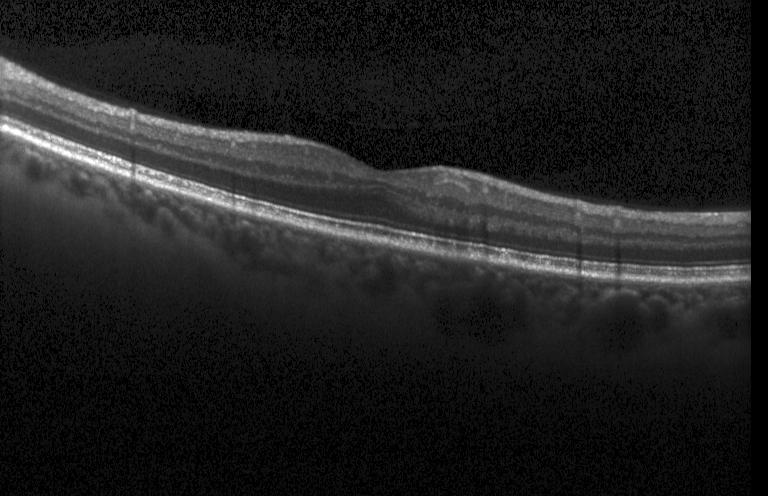
Optical coherence tomography scan. Diagnosis: no choroidal neovascularization, no diabetic macular edema, and no drusen.